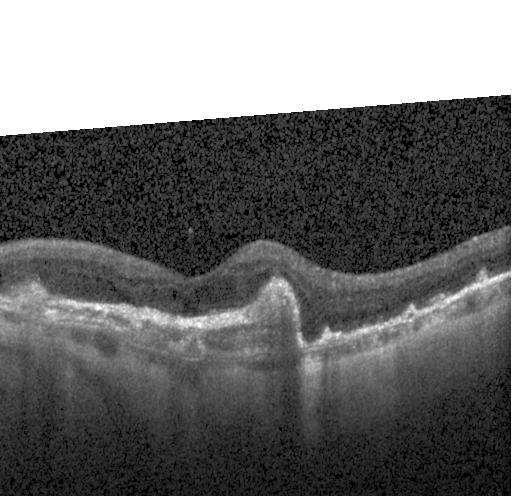

Retinal OCT B-scan.
A choroidal neovascular membrane.